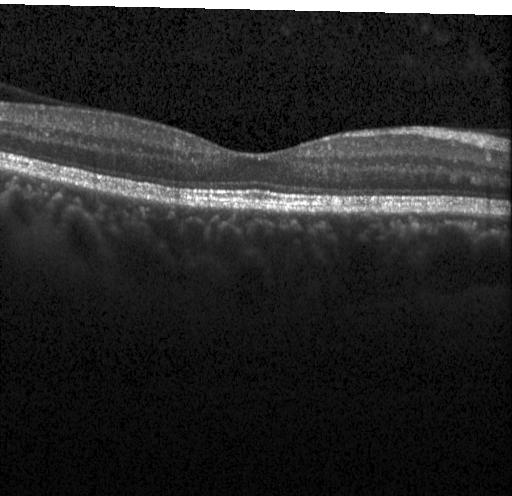
Optical coherence tomography B-scan · instrument: Heidelberg Spectralis · fovea-centered — Assessment: no choroidal neovascularization, diabetic macular edema, or drusen.